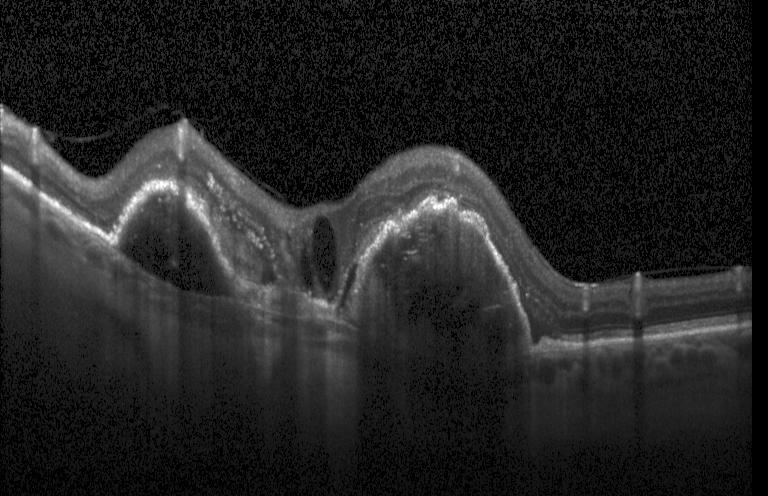 Spectral-domain OCT; optical coherence tomography B-scan; fovea-centered; instrument: Heidelberg Spectralis — Assessment: choroidal neovascularization (CNV).